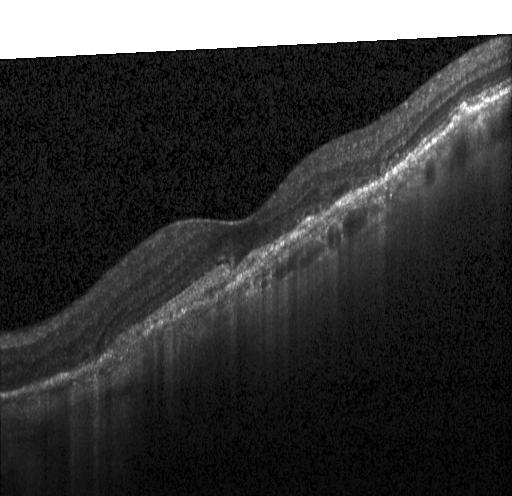

OCT line scan. Macular scan. Spectral-domain OCT — Dx: choroidal neovascularization (CNV).